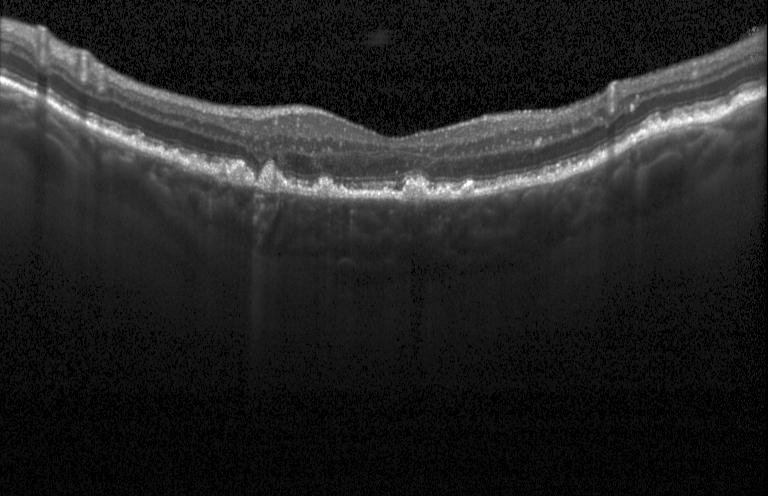

OCT line scan; Heidelberg Spectralis.
A choroidal neovascular membrane.